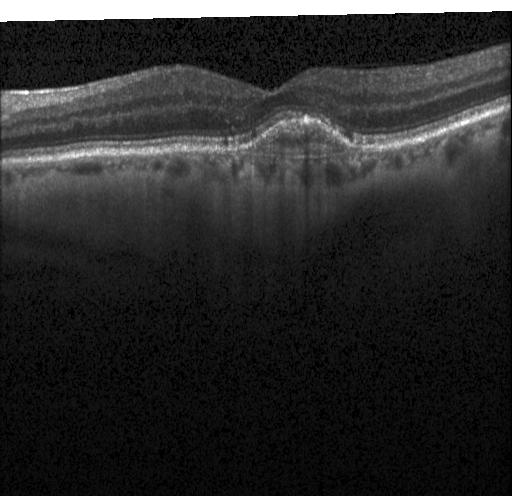

Spectral-domain optical coherence tomography; OCT line scan; fovea-centered — Finding: choroidal neovascularization.